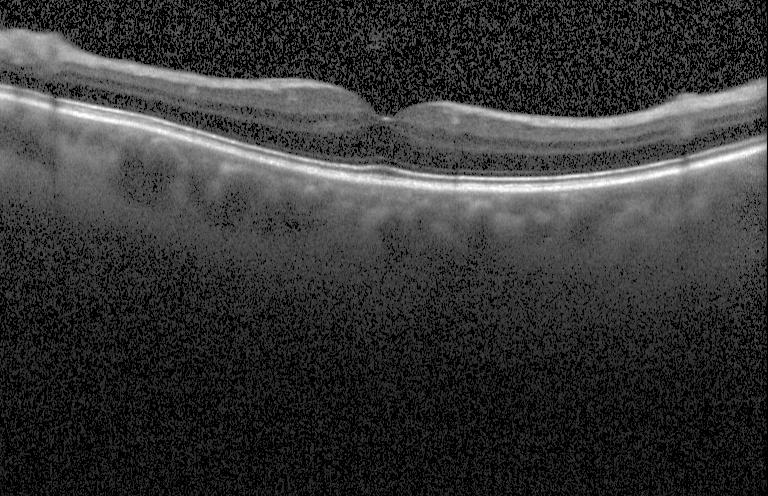
Finding: no evidence of choroidal neovascularization, diabetic macular edema, or drusen.